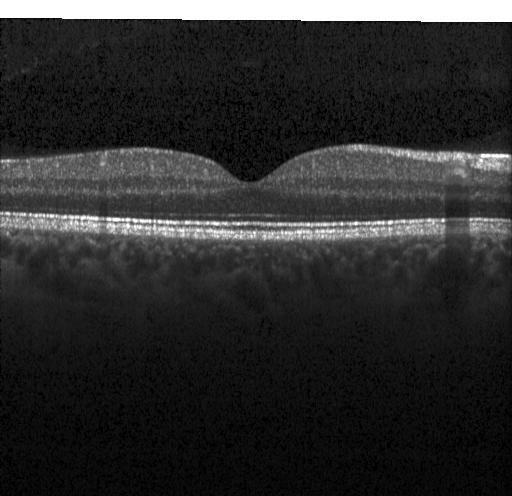 Macular scan, retinal OCT cross-section, acquired on a Heidelberg Spectralis, spectral-domain OCT — OCT finding: no choroidal neovascularization, diabetic macular edema, or drusen.